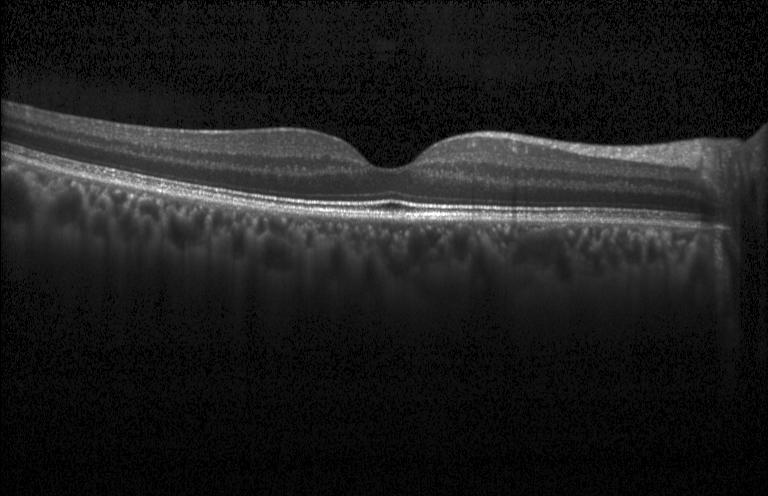
Heidelberg Spectralis · horizontal scan through the fovea · spectral-domain OCT · OCT B-scan. Macular OCT: no evidence of choroidal neovascularization, diabetic macular edema, or drusen.